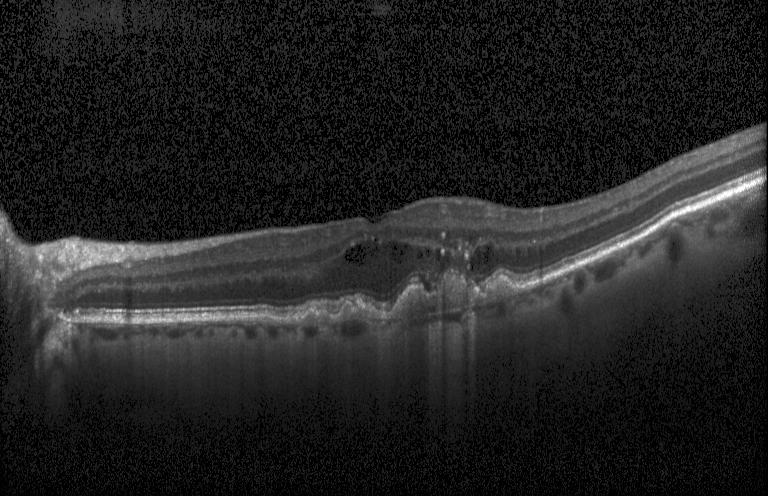

Macular OCT: a choroidal neovascular membrane.